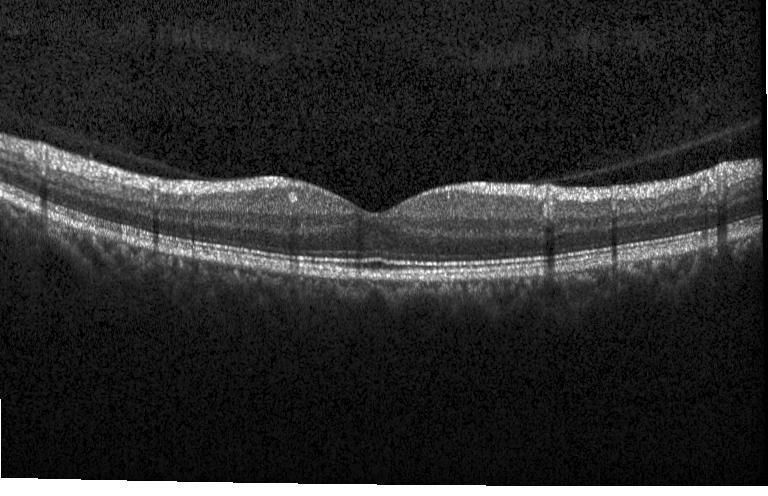 Macular OCT: neither choroidal neovascularization, diabetic macular edema, nor drusen.